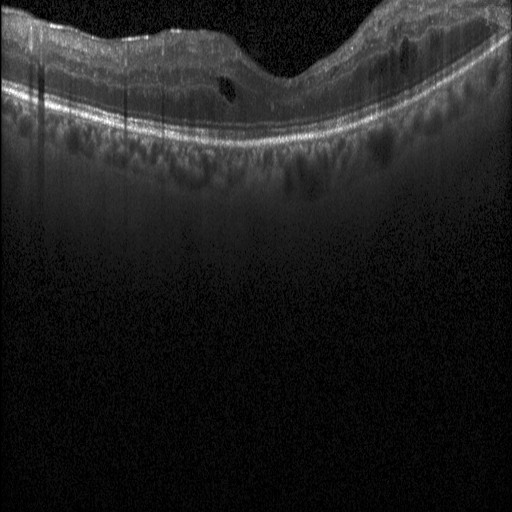 OCT line scan, centered on the fovea. Assessment: diabetic macular edema (DME).